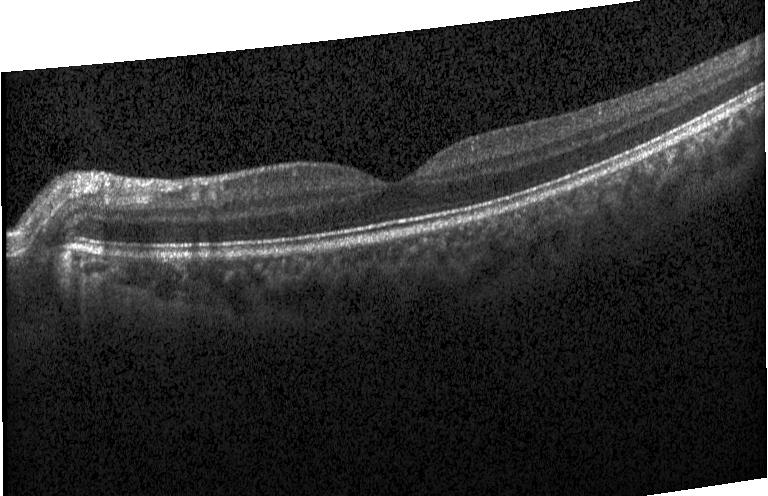 Optical coherence tomography B-scan · horizontal scan through the fovea · spectral-domain optical coherence tomography.
The scan shows no CNV, DME, or drusen.